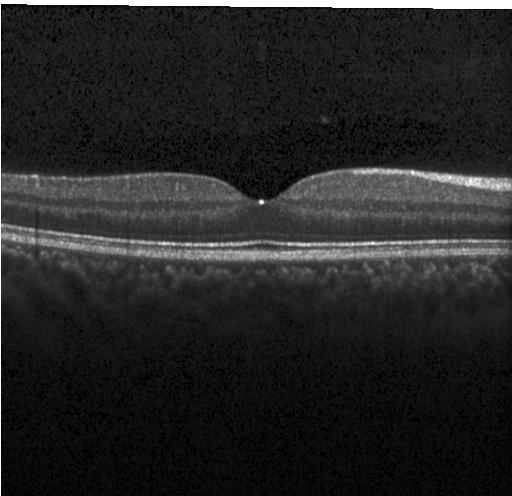 Retinal OCT cross-section. Diagnosis: no evidence of choroidal neovascularization, diabetic macular edema, or drusen.